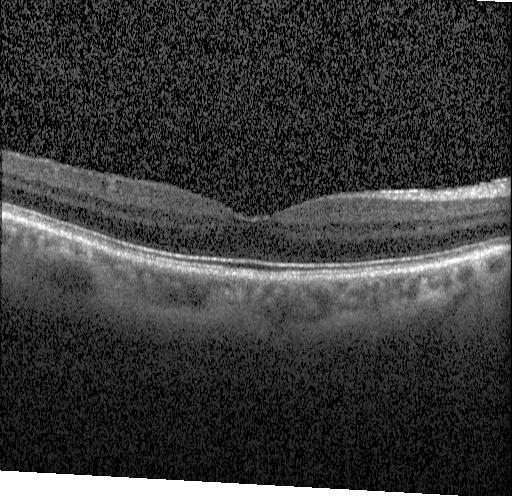
Diagnosis: no CNV, DME, or drusen.